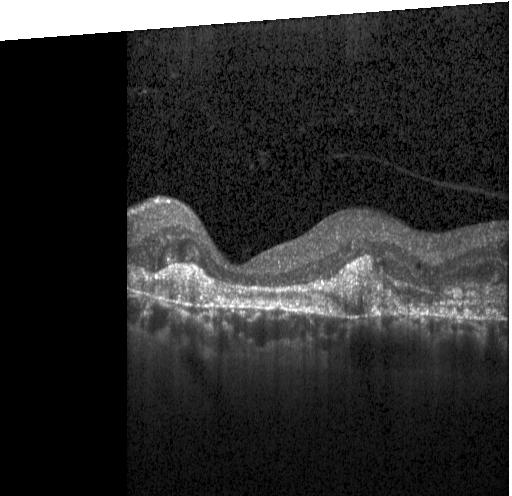

Horizontal scan through the fovea. Retinal OCT cross-section — Diagnosis: choroidal neovascularization (CNV).